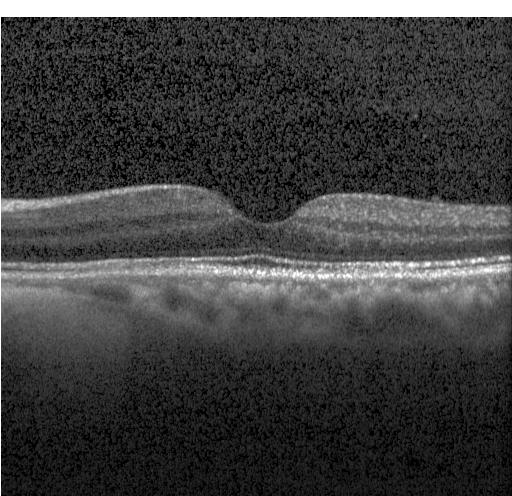

Diagnosis: no CNV, no DME, and no drusen.